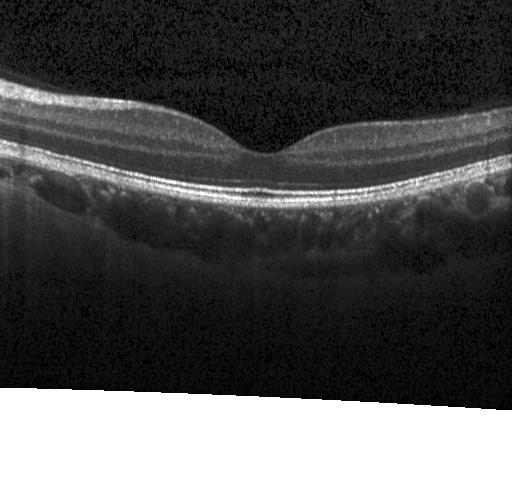
No CNV, no DME, and no drusen.